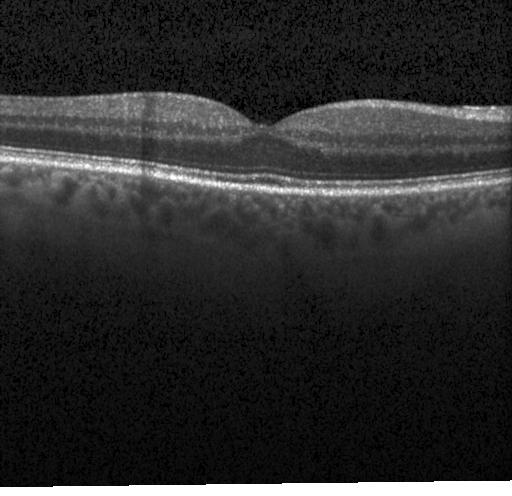
Horizontal scan through the fovea; Heidelberg Spectralis OCT system; spectral-domain optical coherence tomography; OCT B-scan — Diagnosis: neither CNV, DME, nor drusen.